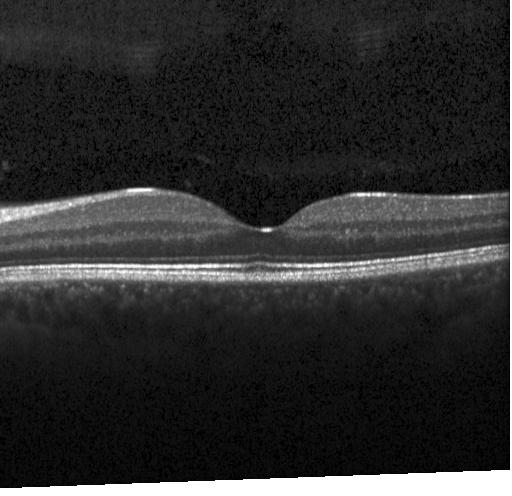 Through the macula, retinal OCT cross-section, acquired on a Heidelberg Spectralis, spectral-domain OCT.
Macular OCT: no evidence of choroidal neovascularization, diabetic macular edema, or drusen.